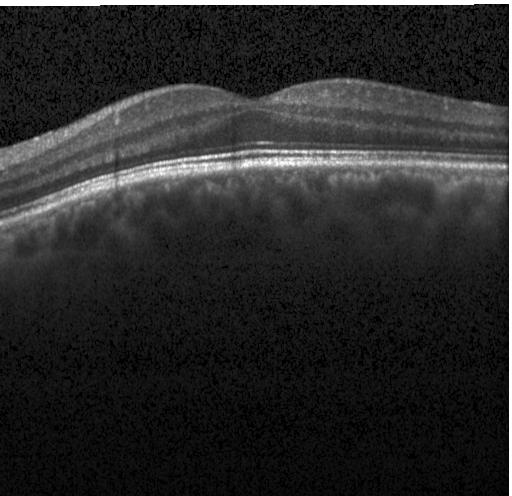
No CNV, DME, or drusen.